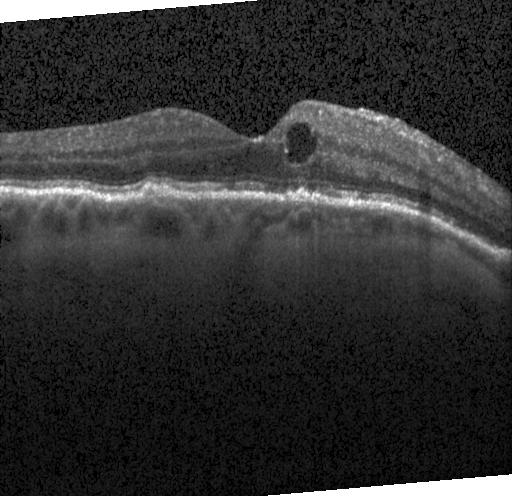

Macular OCT: a choroidal neovascular membrane.